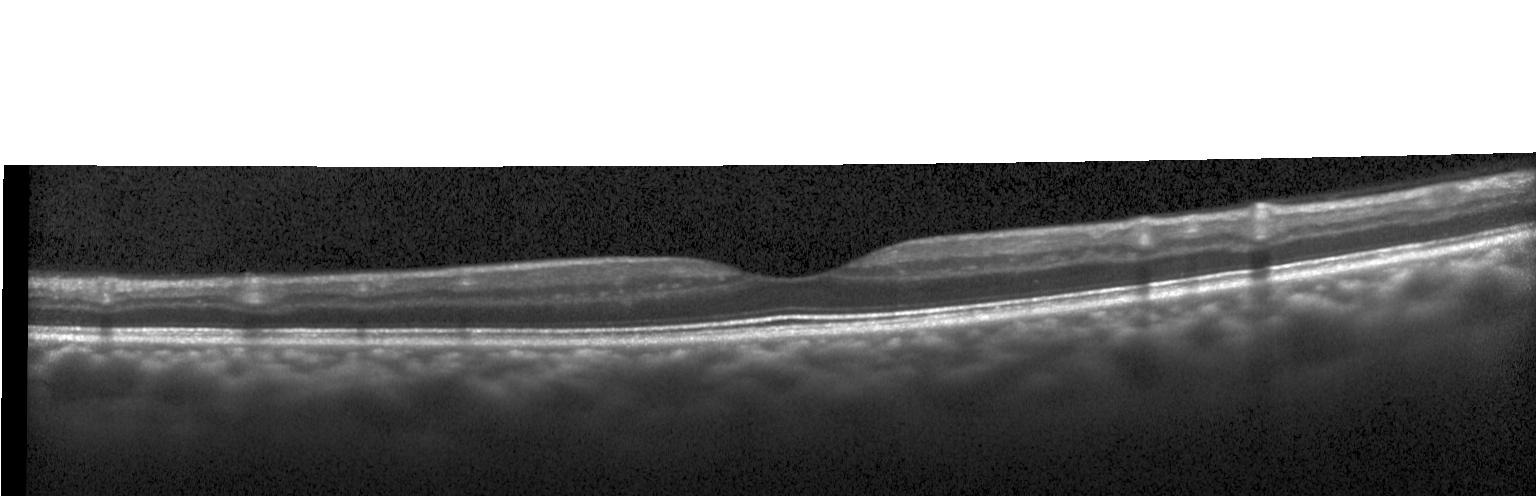
Impression: no choroidal neovascularization, no diabetic macular edema, and no drusen.